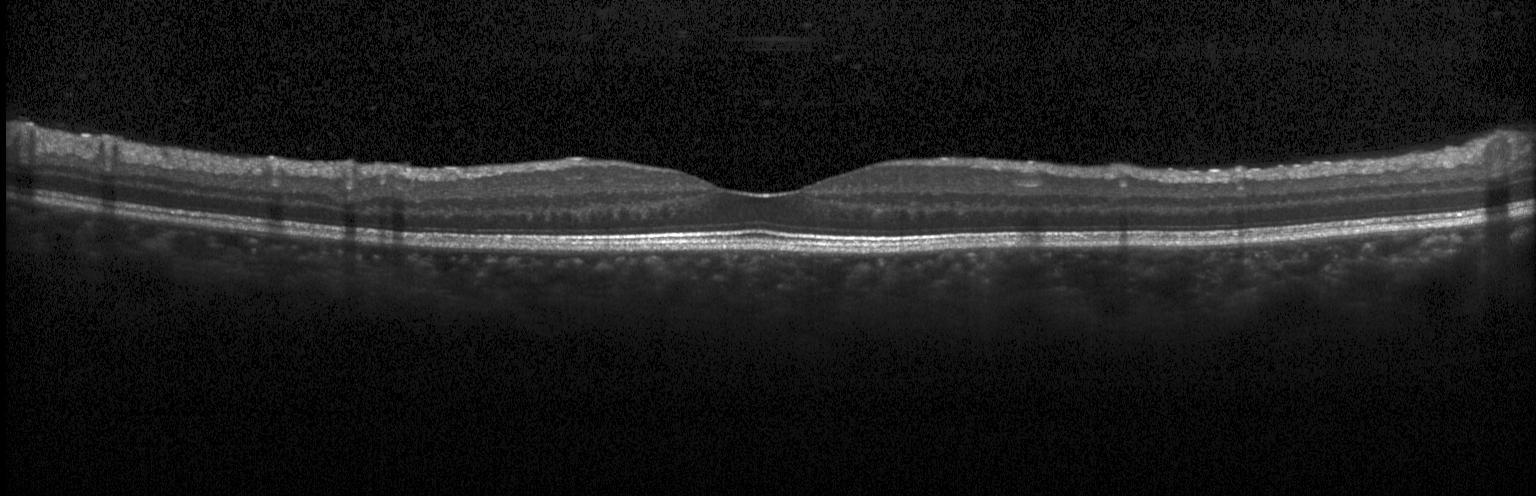

OCT B-scan.
Impression: neither choroidal neovascularization, diabetic macular edema, nor drusen.